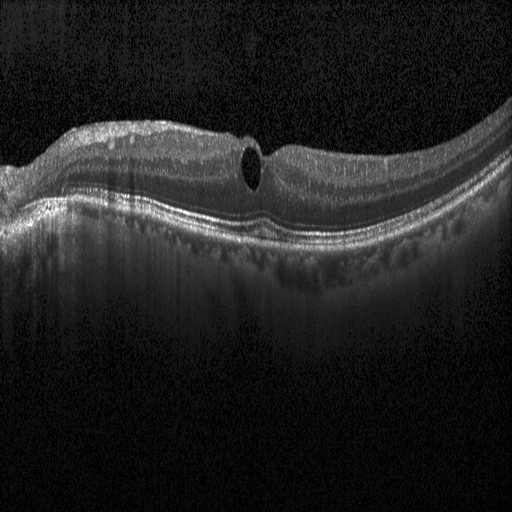 Macular OCT: diabetic macular edema (DME).